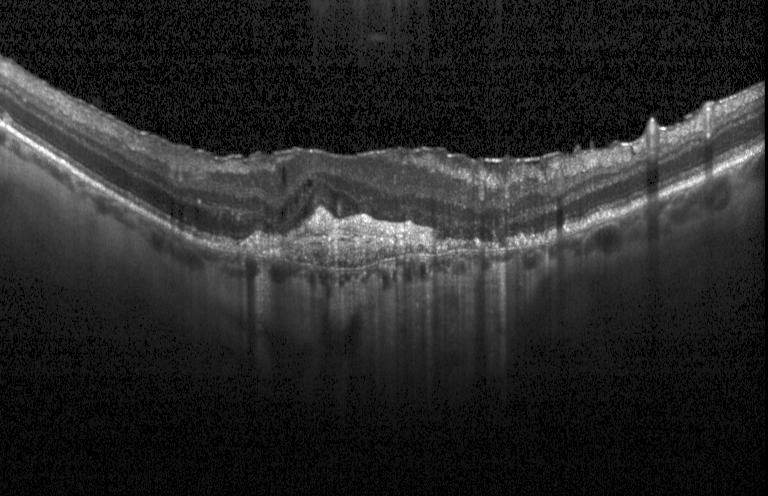 Heidelberg Spectralis. Fovea-centered. Spectral-domain optical coherence tomography. OCT line scan.
Diagnosis: a choroidal neovascular membrane.